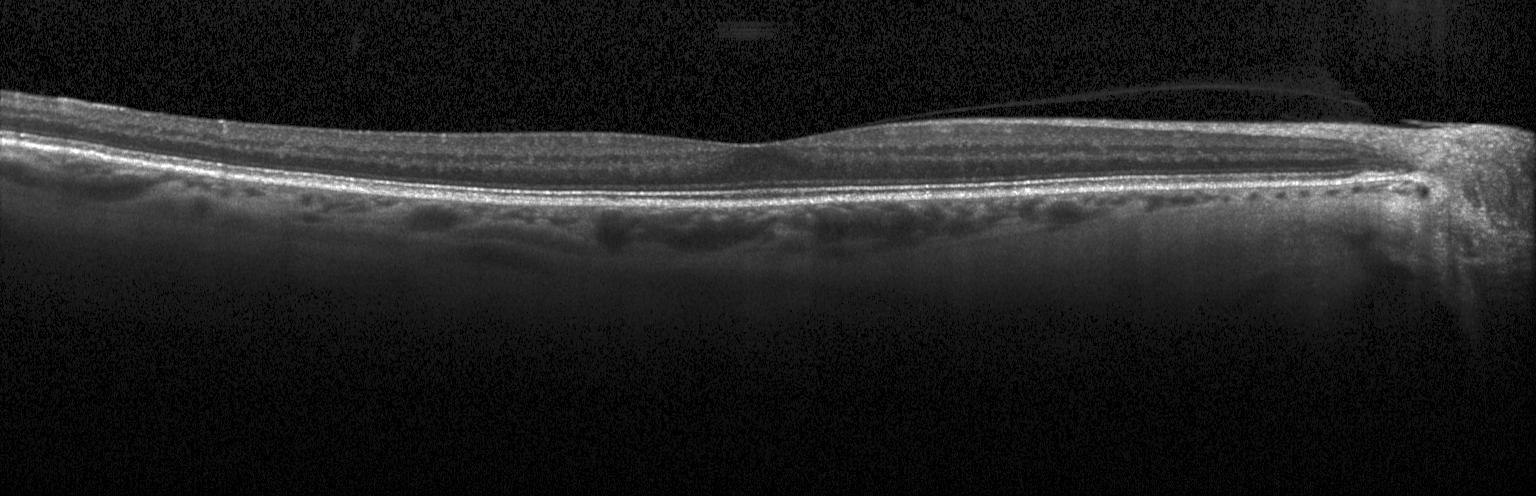 Dx: neither choroidal neovascularization, diabetic macular edema, nor drusen.